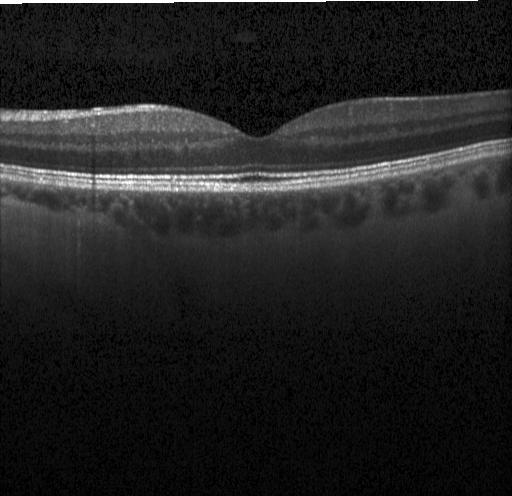
Retinal OCT cross-section · centered on the fovea · SD-OCT.
Finding: no evidence of choroidal neovascularization, diabetic macular edema, or drusen.